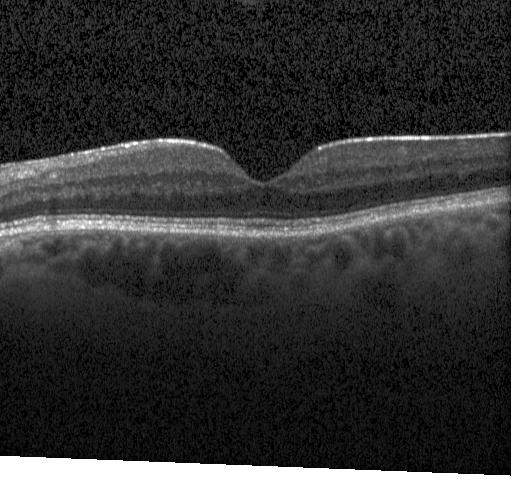
Diagnosis: neither choroidal neovascularization, diabetic macular edema, nor drusen.